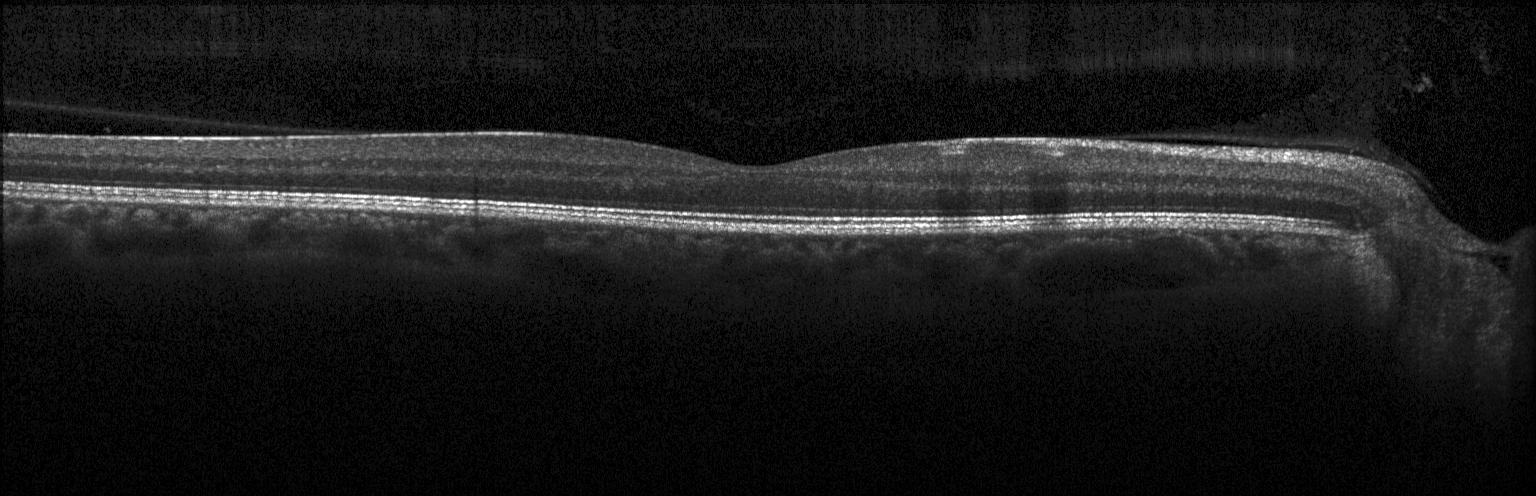 Diagnosis: no evidence of choroidal neovascularization, diabetic macular edema, or drusen.